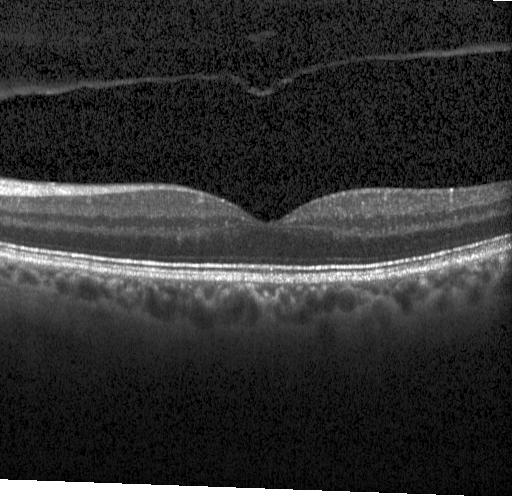
OCT line scan
No choroidal neovascularization, diabetic macular edema, or drusen.